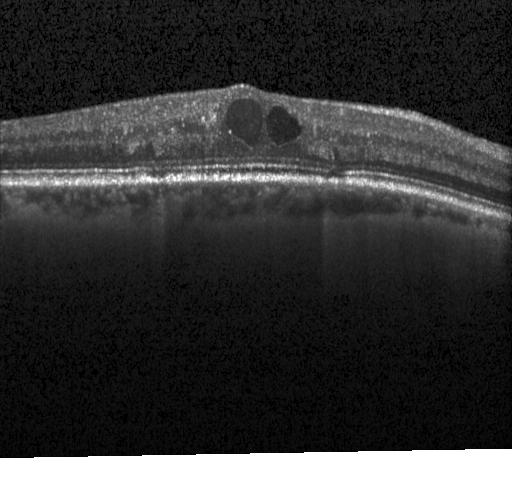 Impression: DME.